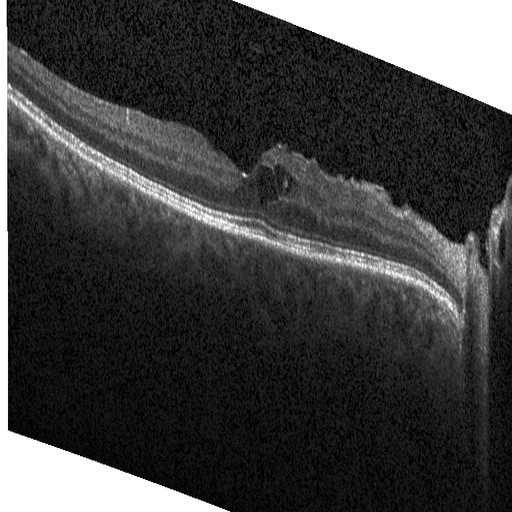

Through the macula · optical coherence tomography B-scan · instrument: Heidelberg Spectralis.
Impression: DME.